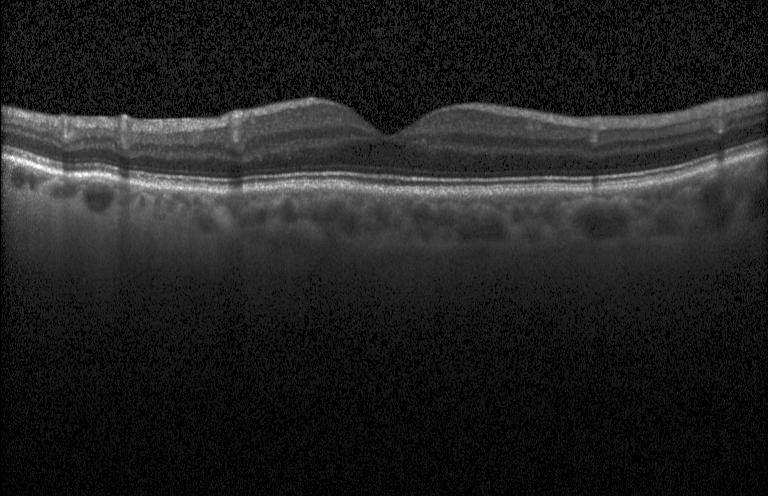

Impression: no evidence of choroidal neovascularization, diabetic macular edema, or drusen.